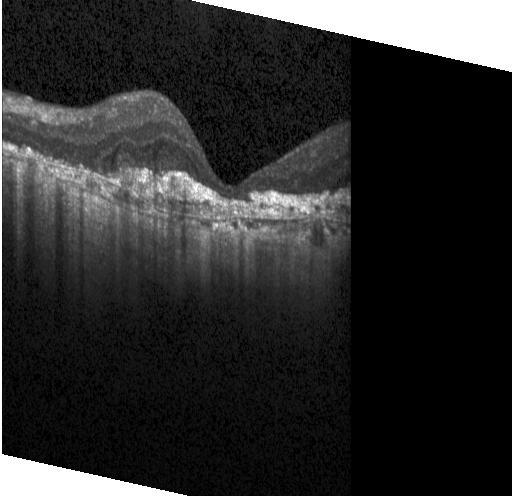

Spectral-domain OCT · acquired on a Heidelberg Spectralis · optical coherence tomography scan.
This B-scan demonstrates a choroidal neovascular membrane.